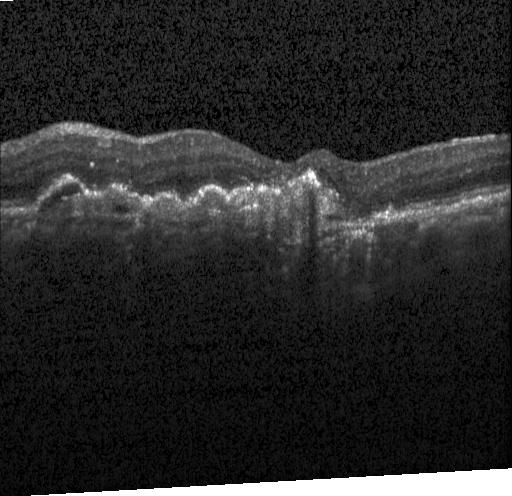 OCT finding: a choroidal neovascular membrane.